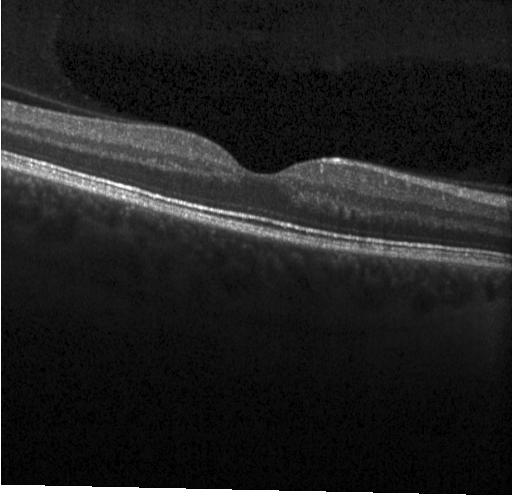 Spectral-domain OCT B-scan: neither choroidal neovascularization, diabetic macular edema, nor drusen.